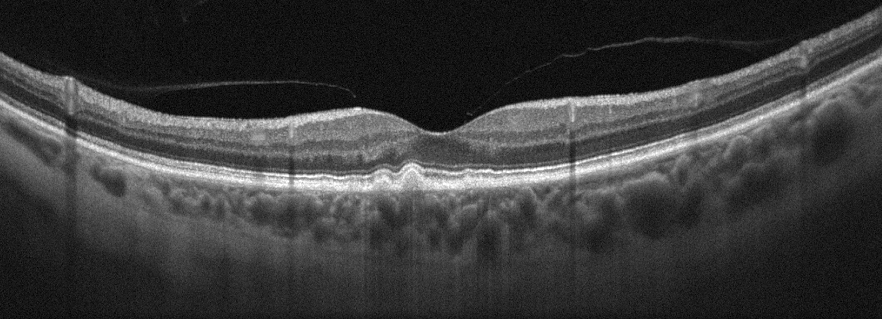
Optovue Avanti RTVue XR; macular scan; optical coherence tomography B-scan.
Diagnosis: age-related macular degeneration.